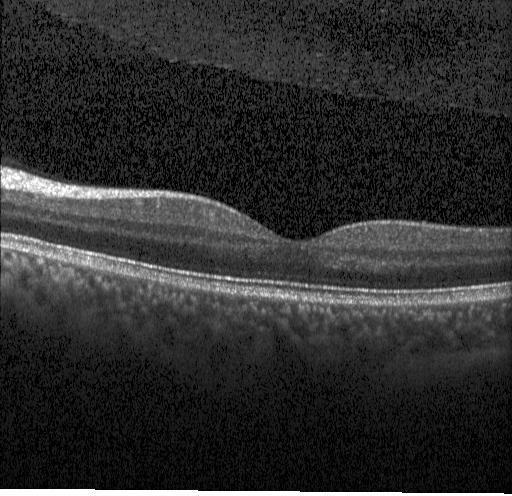
OCT B-scan; SD-OCT — Diagnosis: no choroidal neovascularization, diabetic macular edema, or drusen.